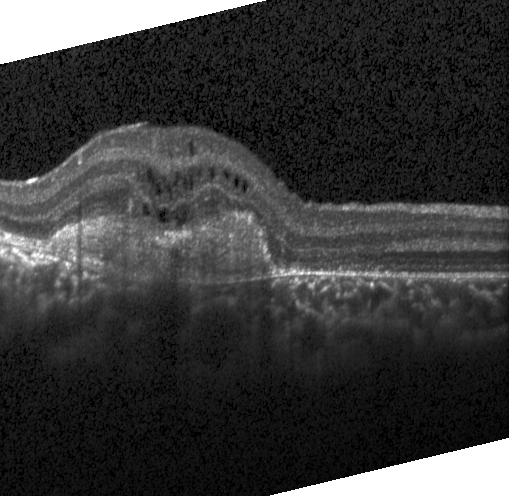 OCT B-scan; spectral-domain OCT; instrument: Heidelberg Spectralis; horizontal scan through the fovea. Assessment: CNV.